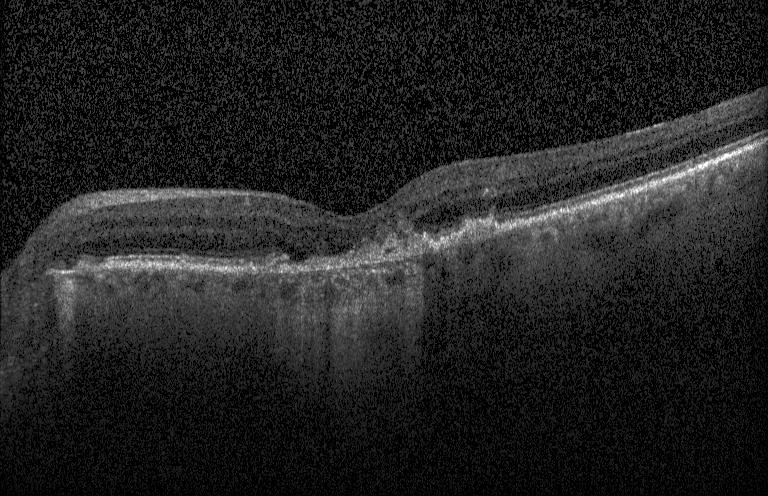
Finding: a choroidal neovascular membrane.